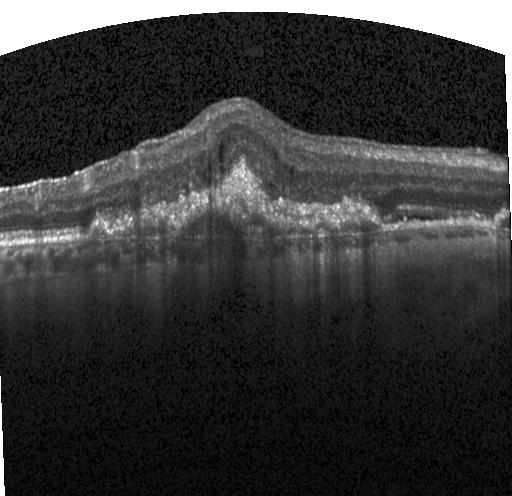
OCT line scan — The scan shows a choroidal neovascular membrane.